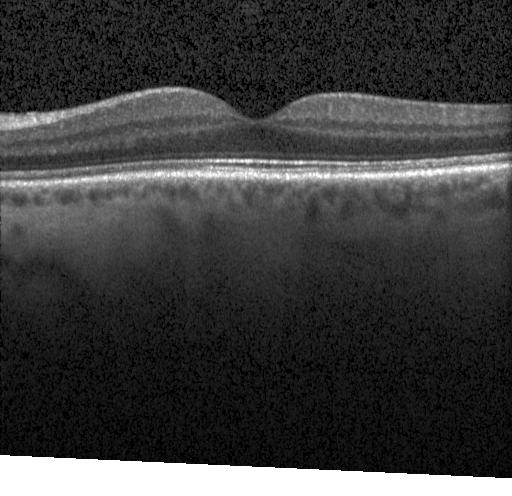
Heidelberg Spectralis, spectral-domain optical coherence tomography, retinal OCT B-scan. Macular OCT: neither choroidal neovascularization, diabetic macular edema, nor drusen.